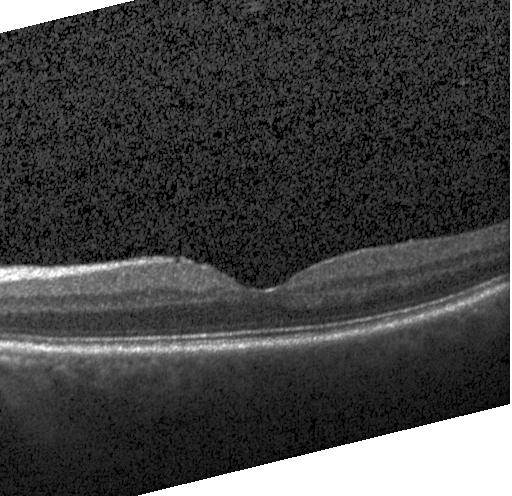
OCT line scan. Spectral-domain optical coherence tomography. Fovea-centered
Assessment: no choroidal neovascularization, diabetic macular edema, or drusen.